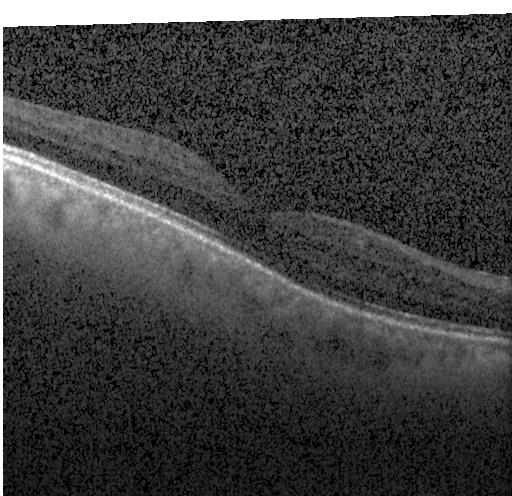

OCT B-scan.
Finding: no evidence of choroidal neovascularization, diabetic macular edema, or drusen.